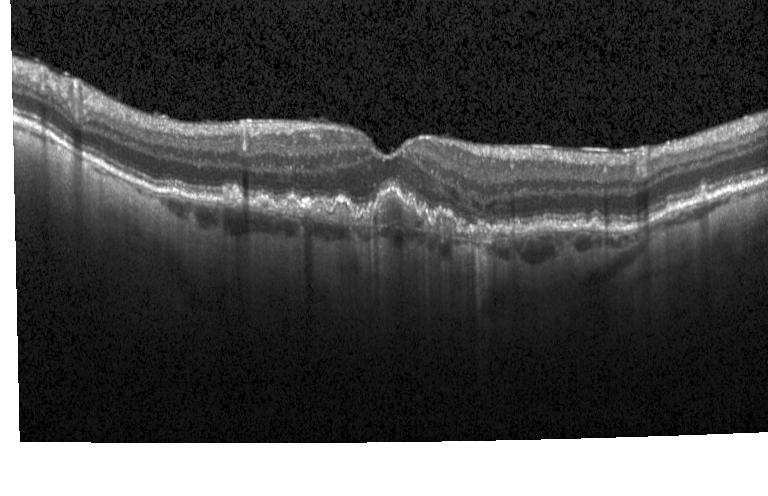
Dx: choroidal neovascularization.